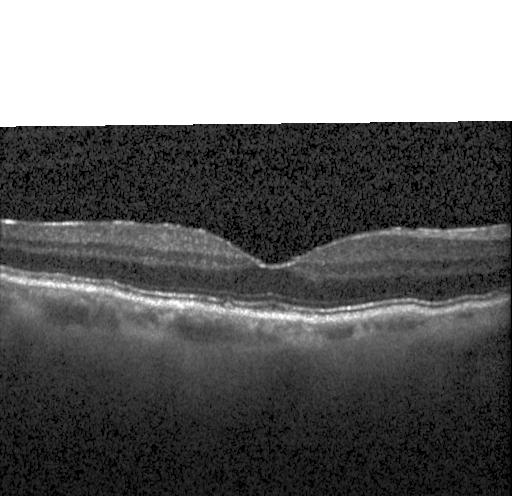 Spectral-domain optical coherence tomography; OCT B-scan — Impression: no CNV, no DME, and no drusen.